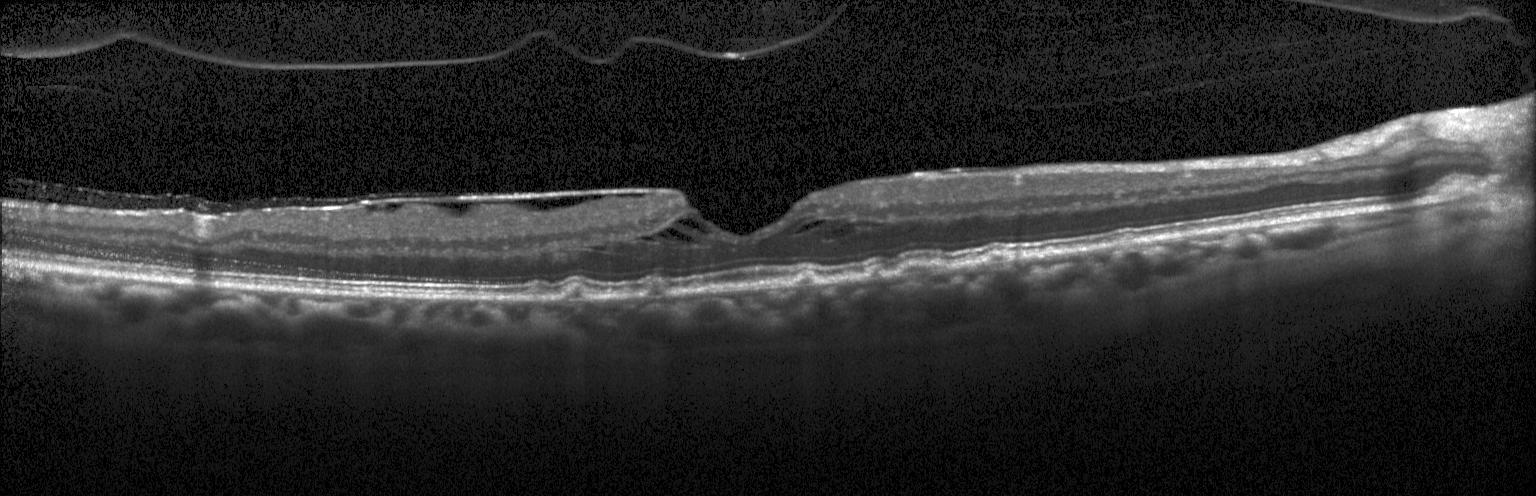 OCT line scan. Macular scan.
Impression: multiple drusen.